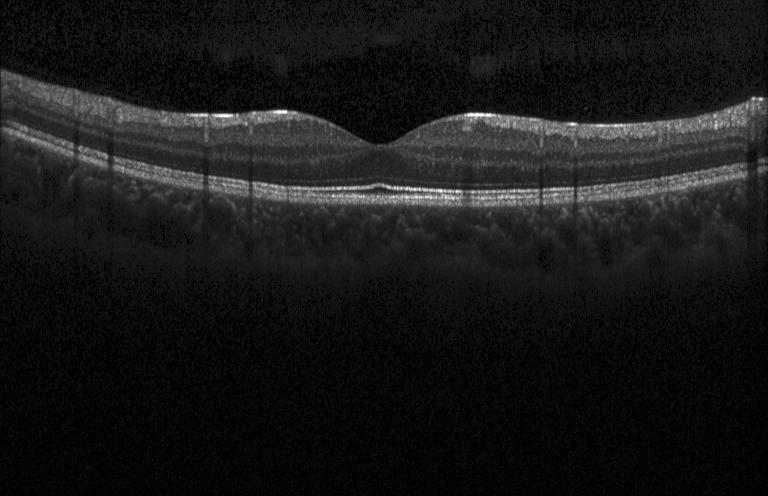
Diagnosis: no CNV, DME, or drusen.